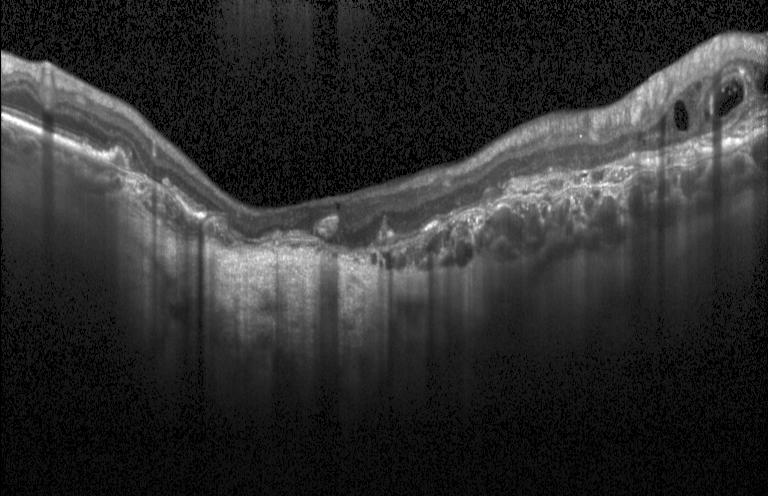

Impression: a choroidal neovascular membrane.